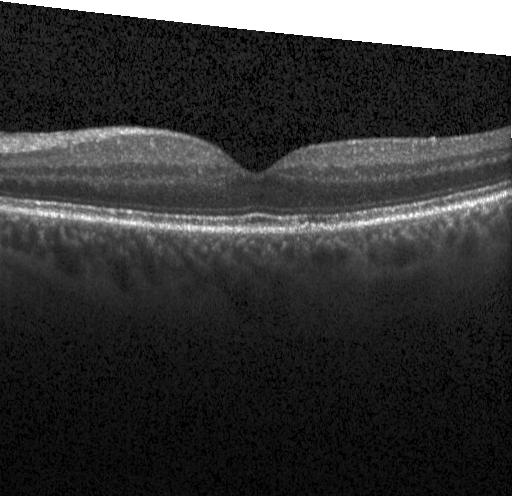 The scan shows no evidence of choroidal neovascularization, diabetic macular edema, or drusen.